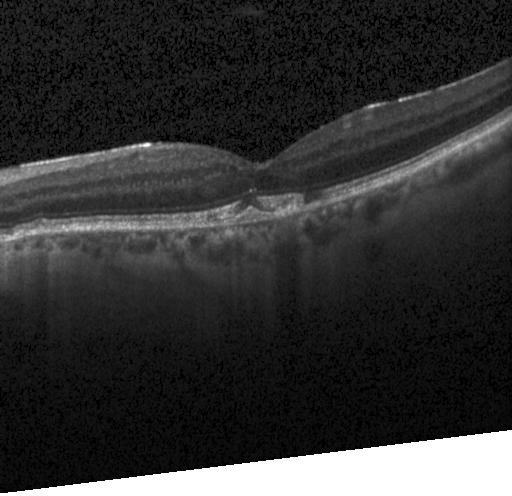
Spectral-domain OCT. Acquired on a Heidelberg Spectralis. Optical coherence tomography B-scan. Through the macula
Assessment: choroidal neovascularization (CNV).